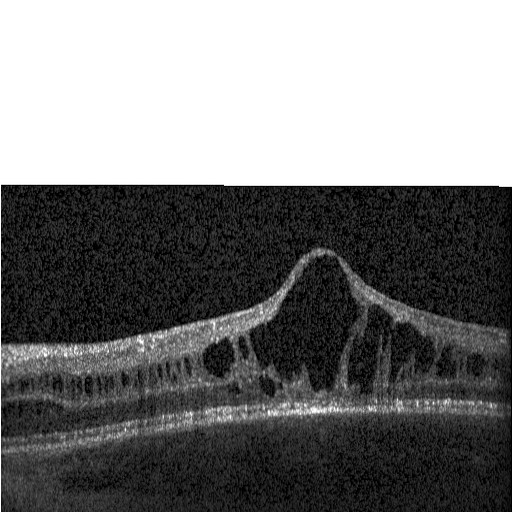

Instrument: Heidelberg Spectralis. Spectral-domain OCT. Macular scan. Optical coherence tomography B-scan. Diagnosis: DME.